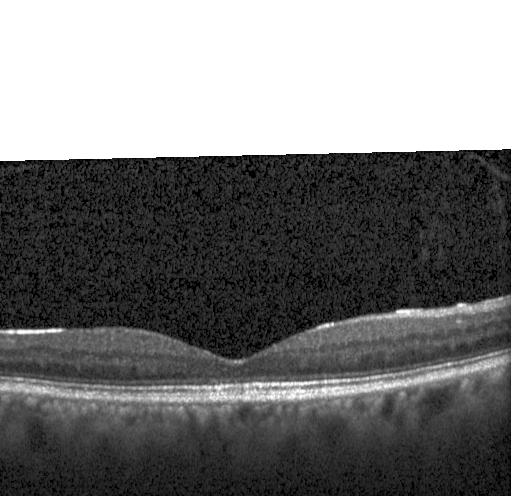
OCT B-scan showing no choroidal neovascularization, no diabetic macular edema, and no drusen.